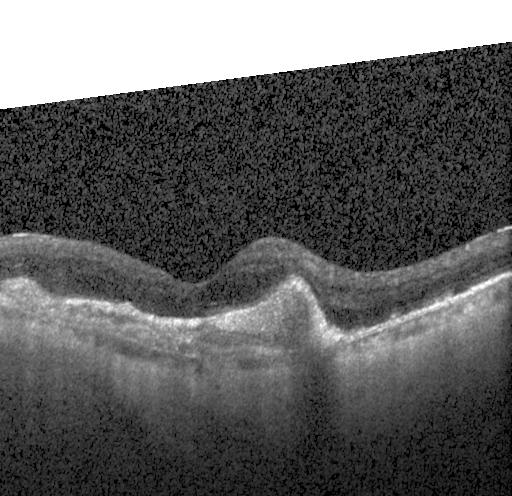 Retinal OCT cross-section, horizontal scan through the fovea. Impression: choroidal neovascularization.